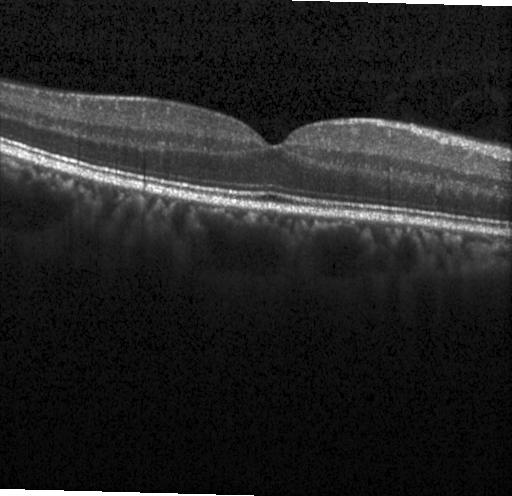
Optical coherence tomography B-scan, fovea-centered, spectral-domain optical coherence tomography, acquired on a Heidelberg Spectralis.
Finding: no choroidal neovascularization, no diabetic macular edema, and no drusen.